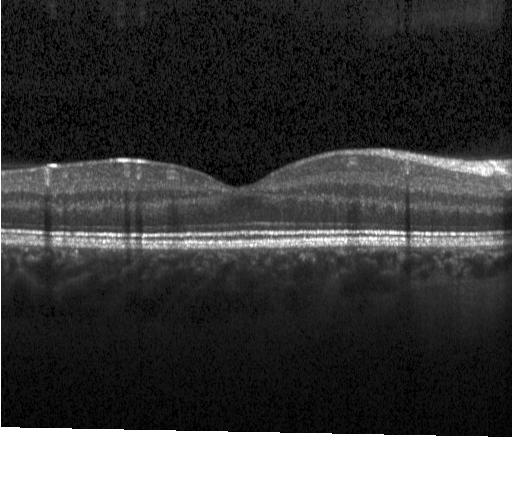
Optical coherence tomography scan — Diagnosis: no choroidal neovascularization, no diabetic macular edema, and no drusen.